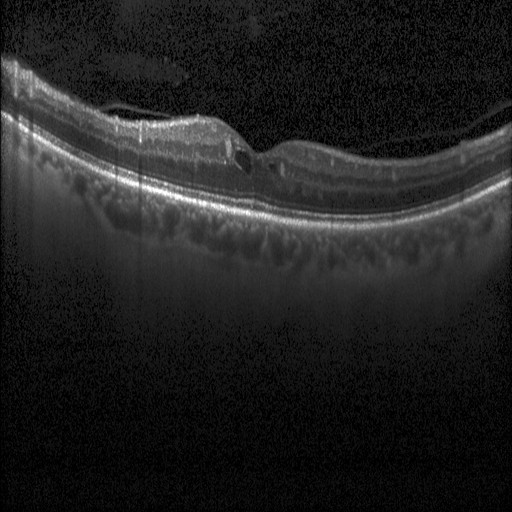

OCT finding: DME.